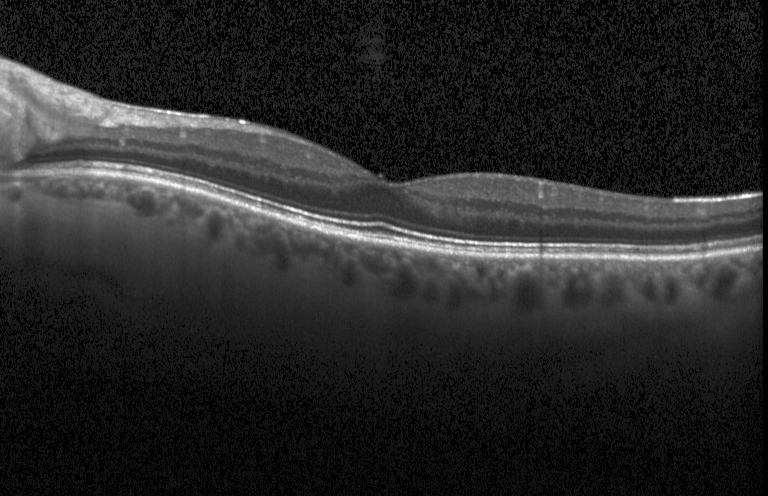
OCT scan showing no choroidal neovascularization, no diabetic macular edema, and no drusen.